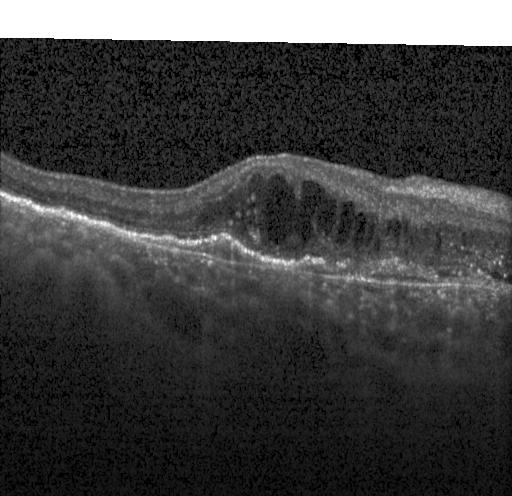

Instrument: Heidelberg Spectralis, through the macula, retinal OCT B-scan. A choroidal neovascular membrane.